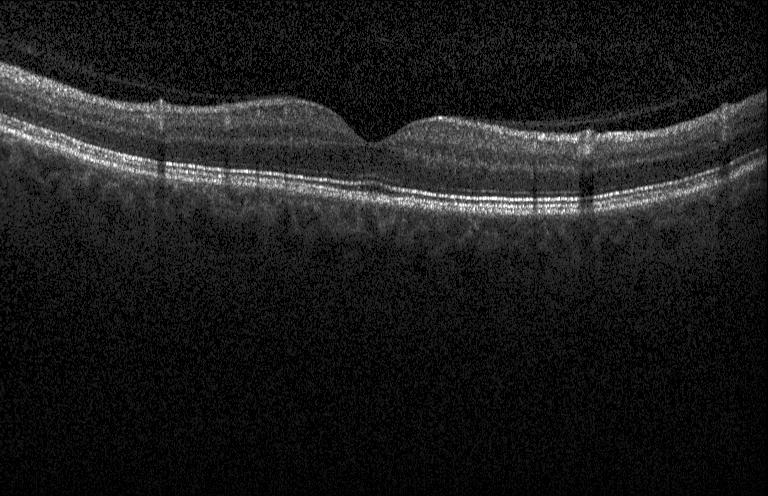

Optical coherence tomography B-scan — Diagnosis: no evidence of choroidal neovascularization, diabetic macular edema, or drusen.